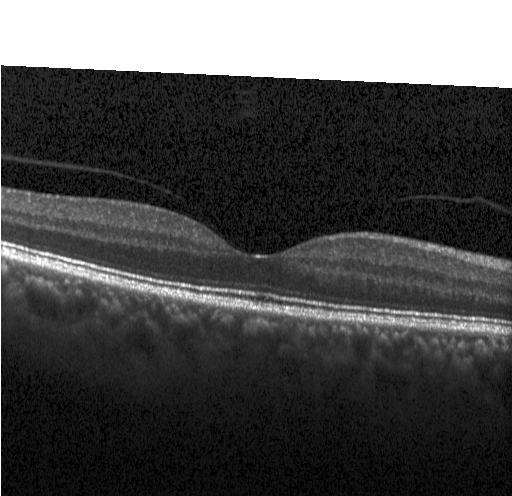
OCT B-scan. Diagnosis: no CNV, no DME, and no drusen.